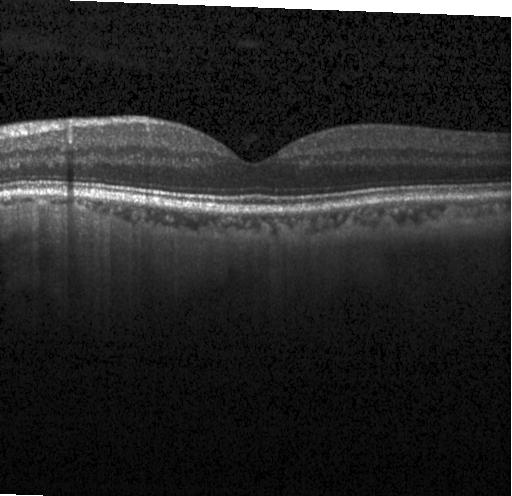 OCT line scan.
No choroidal neovascularization, no diabetic macular edema, and no drusen.